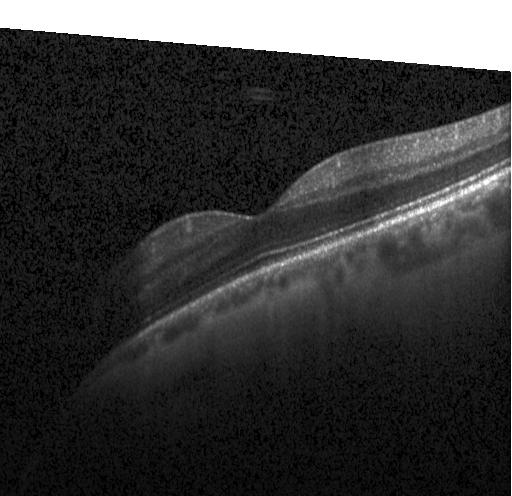

Finding: no choroidal neovascularization, no diabetic macular edema, and no drusen.